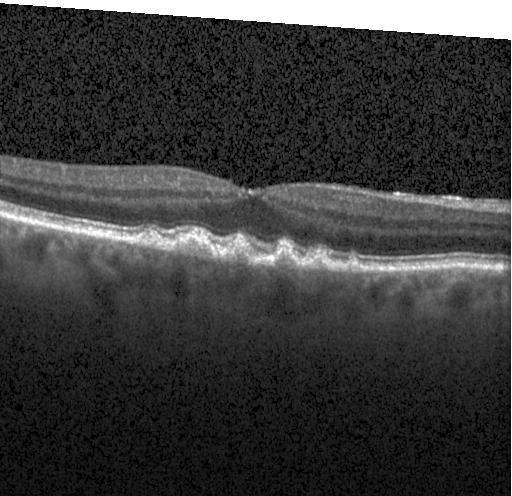 Macular OCT demonstrating sub-RPE drusenoid deposits.